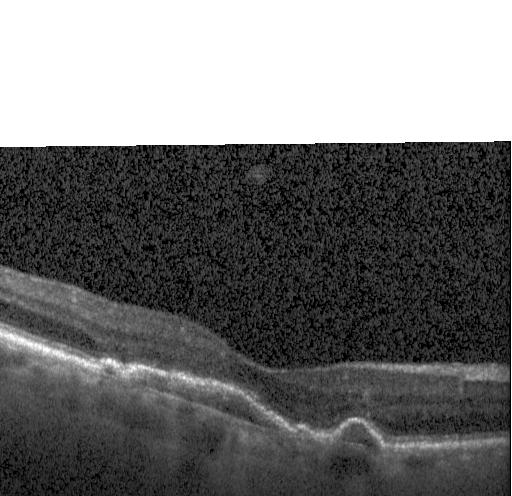 Impression: a choroidal neovascular membrane.